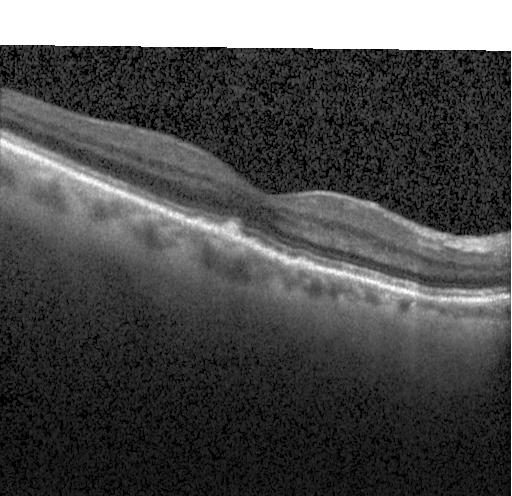

Heidelberg Spectralis OCT system. OCT line scan.
The scan shows sub-RPE drusenoid deposits.